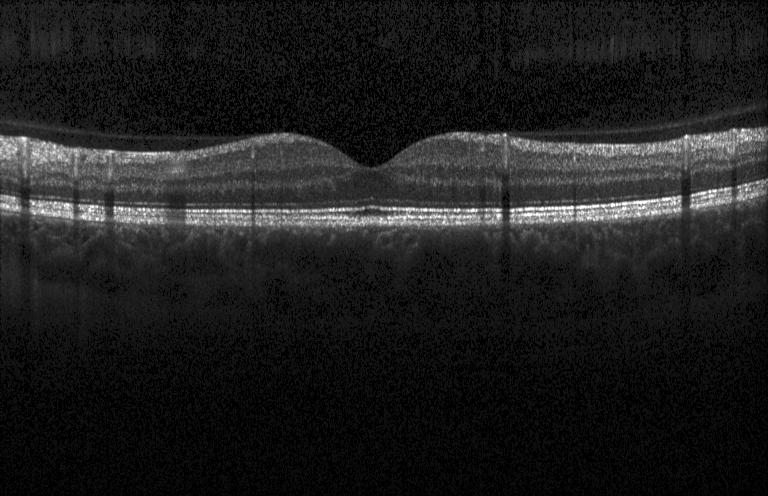 Heidelberg Spectralis, optical coherence tomography scan — Finding: neither choroidal neovascularization, diabetic macular edema, nor drusen.